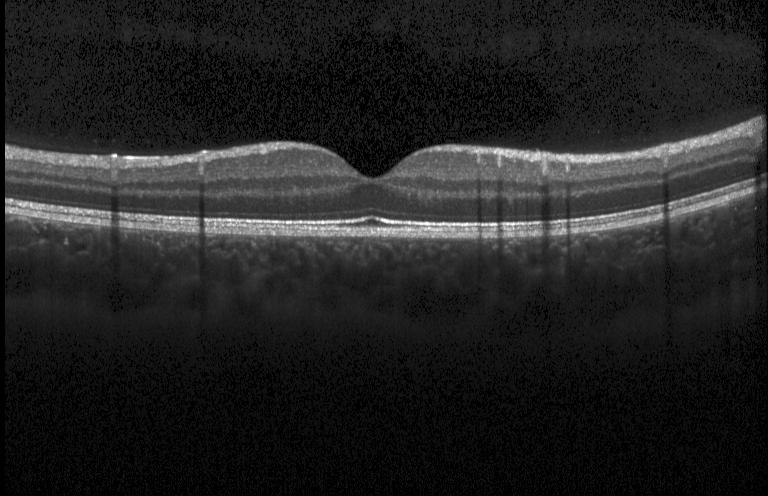
Optical coherence tomography B-scan — Impression: no CNV, no DME, and no drusen.